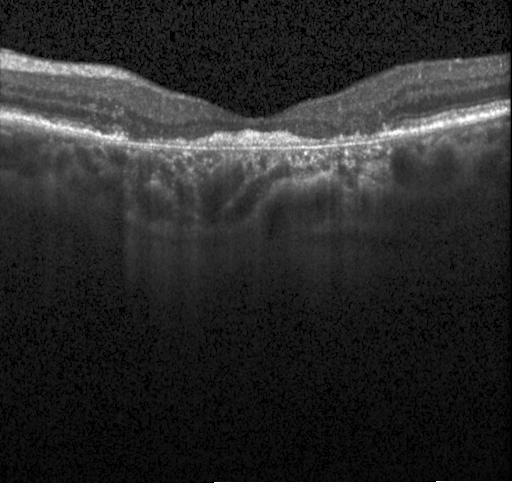 Centered on the fovea · instrument: Heidelberg Spectralis · OCT line scan
Assessment: choroidal neovascularization.